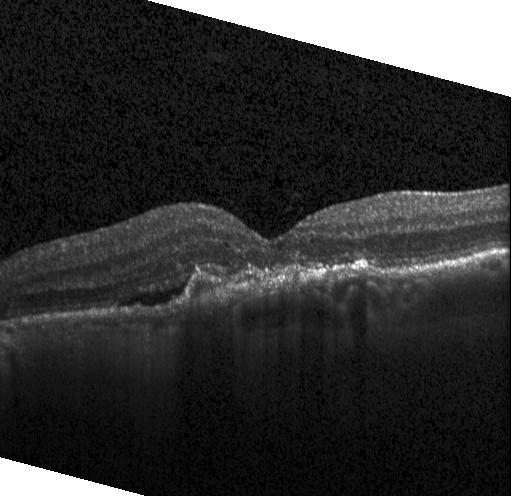 Heidelberg Spectralis OCT system · retinal OCT B-scan. Choroidal neovascularization.